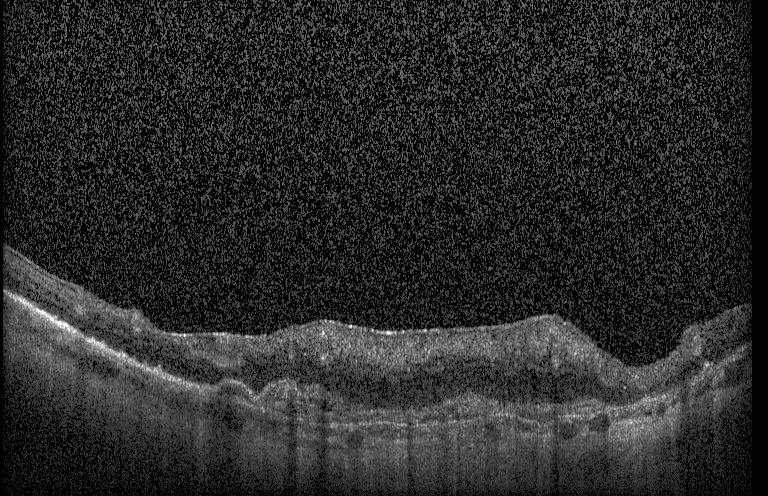 Macular OCT demonstrating CNV.